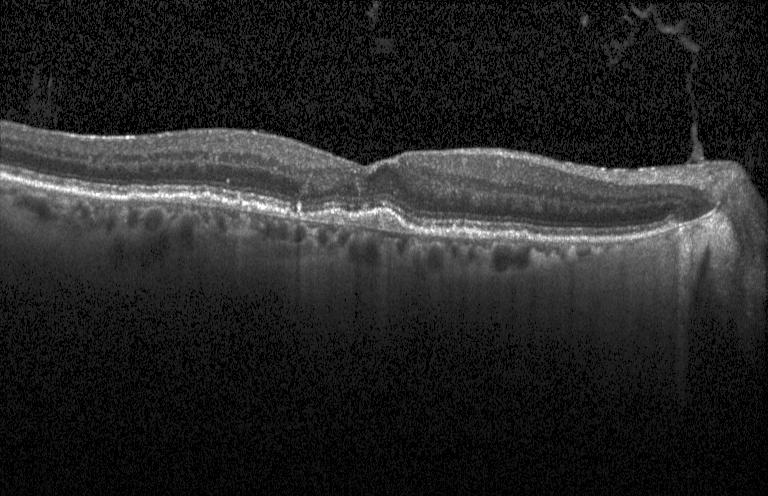 Macular scan. OCT line scan. Spectral-domain optical coherence tomography. Heidelberg Spectralis OCT system — Diagnosis: a choroidal neovascular membrane.